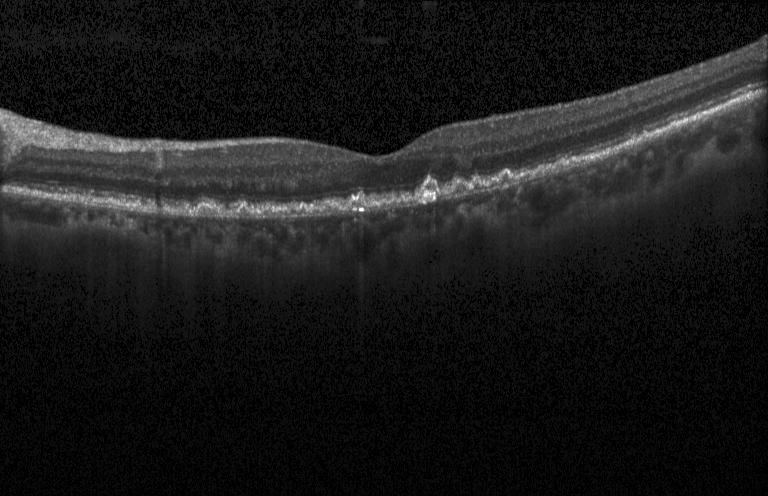 Optical coherence tomography scan, acquired on a Heidelberg Spectralis. Diagnosis: sub-RPE drusenoid deposits.